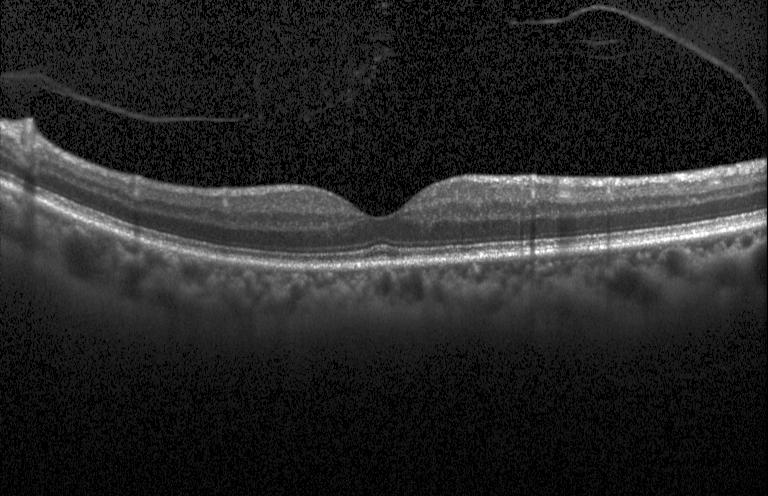

No choroidal neovascularization, diabetic macular edema, or drusen.